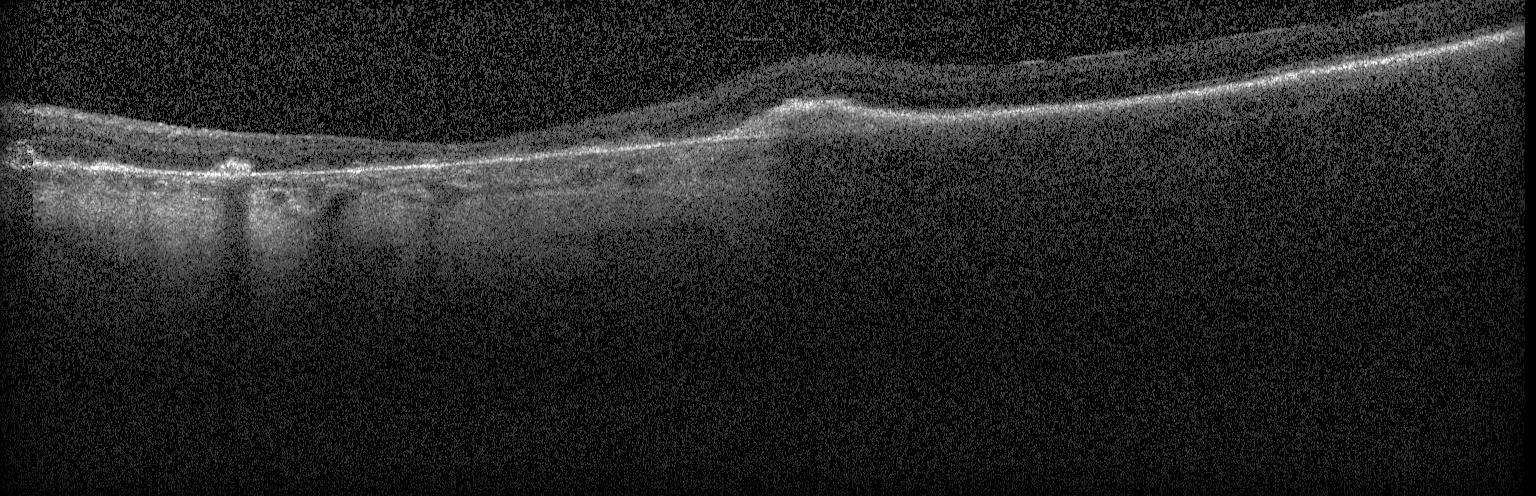

Centered on the fovea · optical coherence tomography scan
OCT finding: a choroidal neovascular membrane.